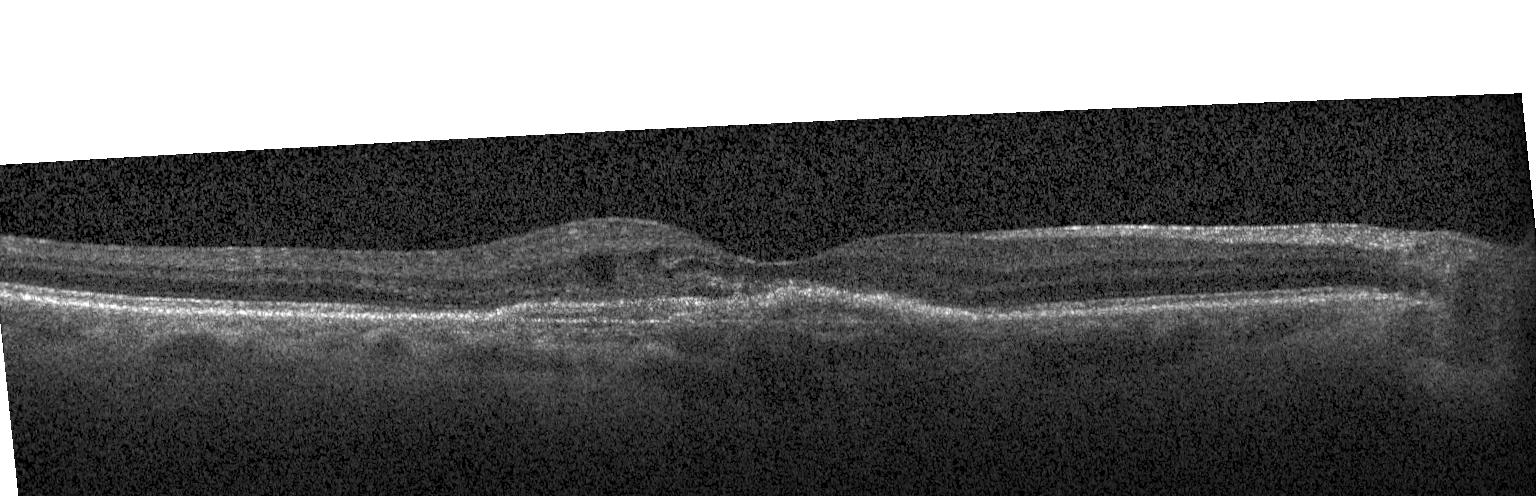
OCT line scan. Instrument: Heidelberg Spectralis. Centered on the fovea. Spectral-domain OCT
Impression: CNV.